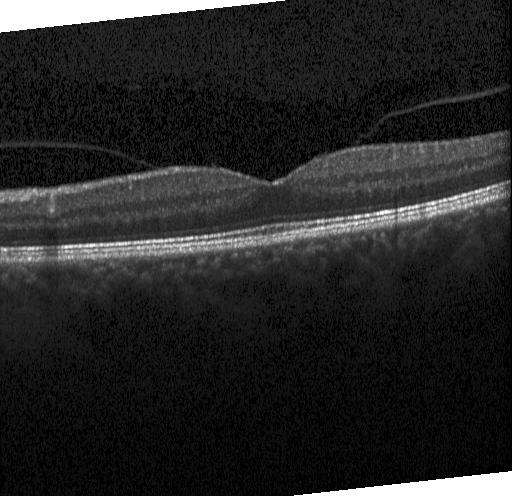

Impression: no choroidal neovascularization, diabetic macular edema, or drusen.